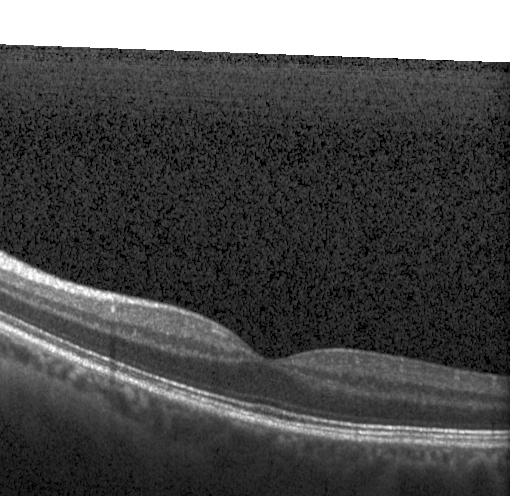
Acquired on a Heidelberg Spectralis, macular scan, OCT B-scan. Diagnosis: no evidence of CNV, DME, or drusen.